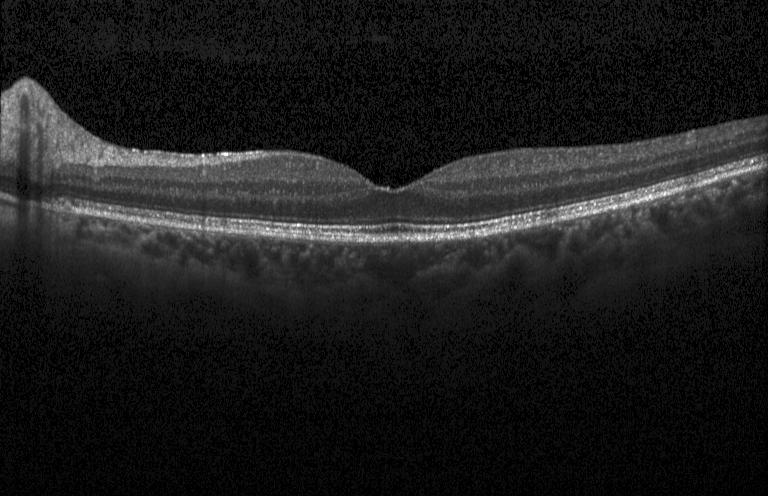
Retinal OCT B-scan — Macular OCT: no evidence of choroidal neovascularization, diabetic macular edema, or drusen.